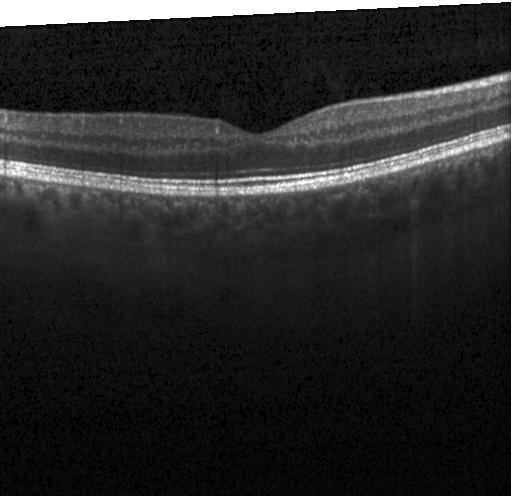

Diagnosis: no choroidal neovascularization, diabetic macular edema, or drusen.